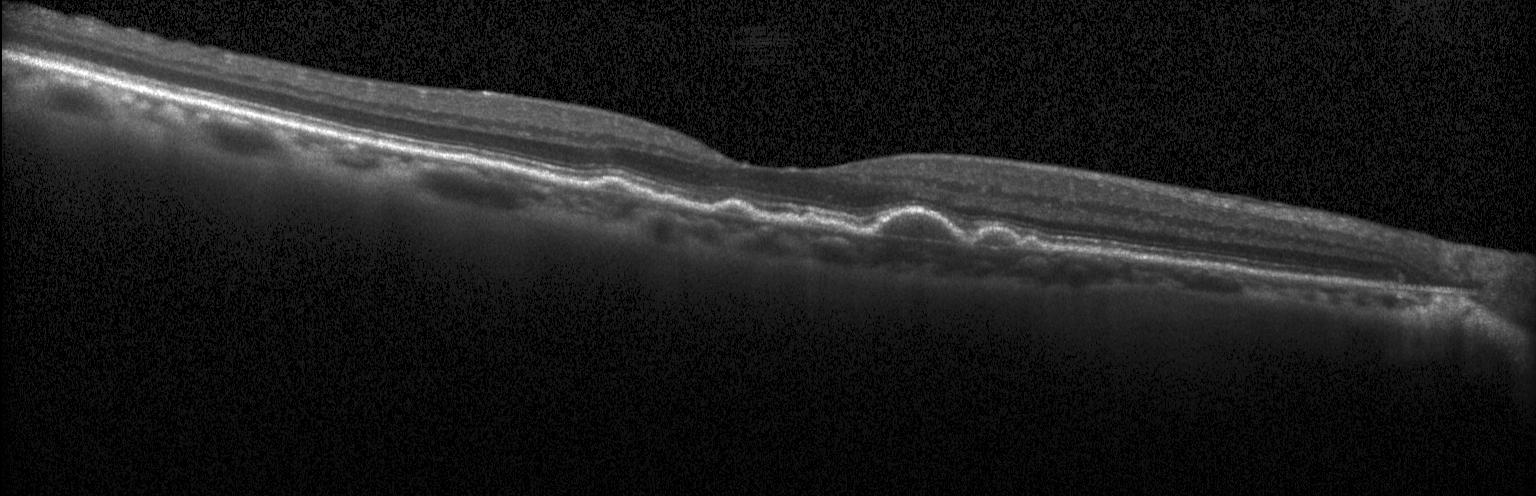
Drusen.